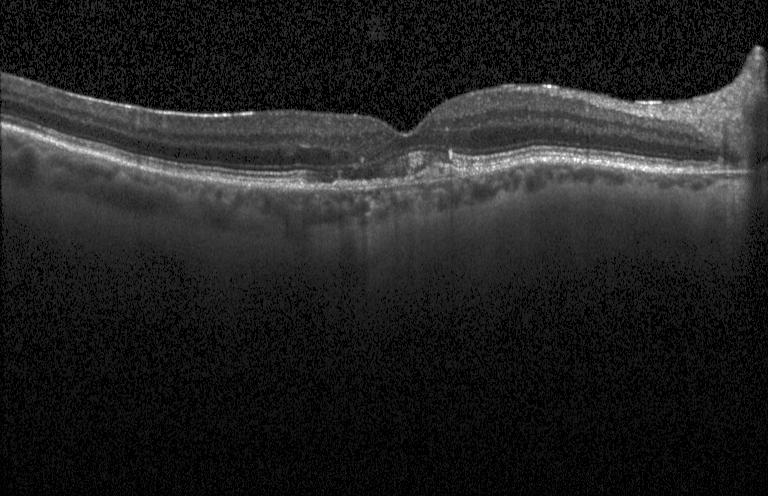
Acquired on a Heidelberg Spectralis · optical coherence tomography scan · SD-OCT · centered on the fovea
Dx: a choroidal neovascular membrane.